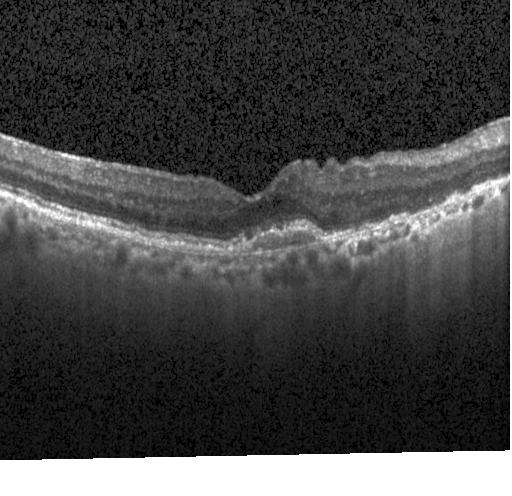

The scan shows a choroidal neovascular membrane.